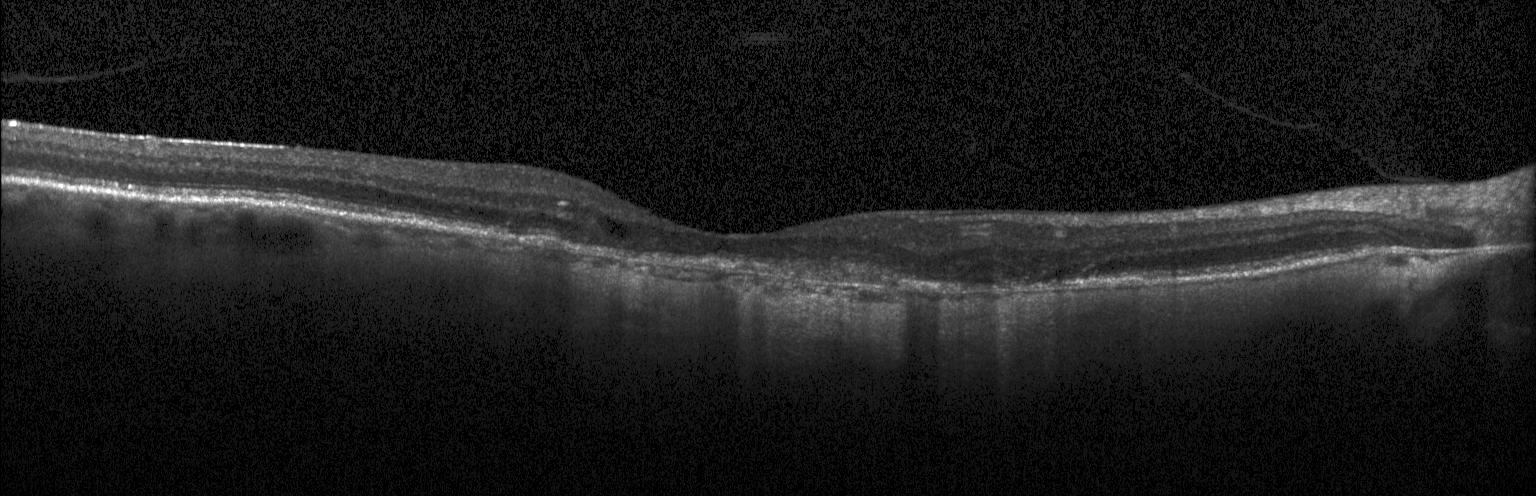
Retinal OCT cross-section, spectral-domain OCT.
Macular OCT: a choroidal neovascular membrane.